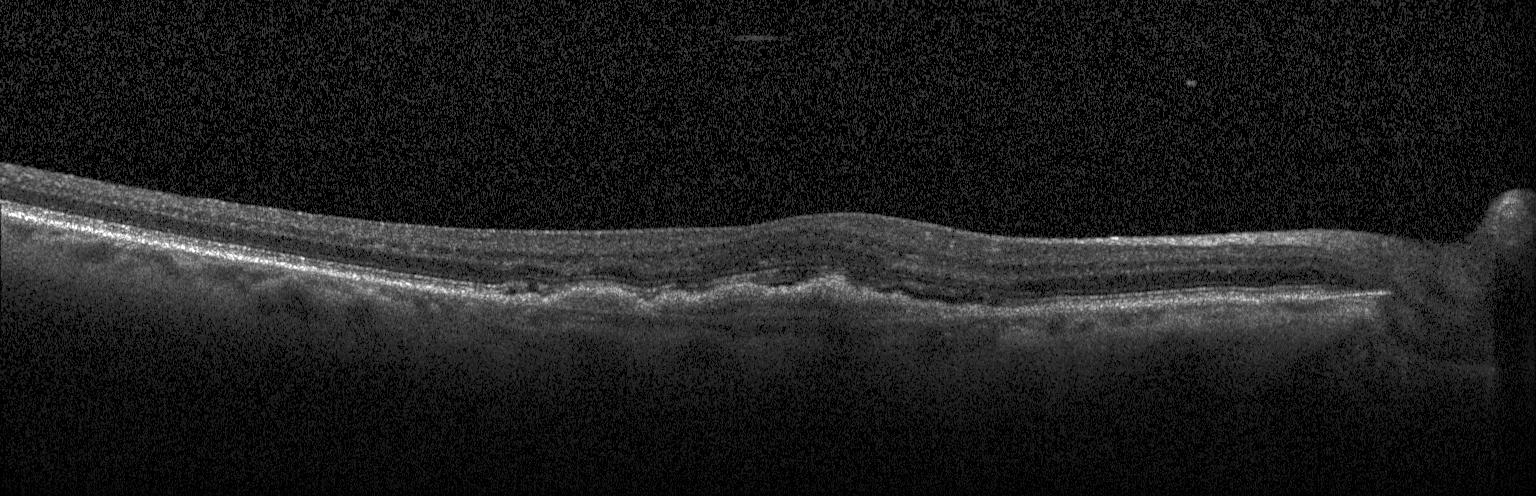 Diagnosis: a choroidal neovascular membrane.